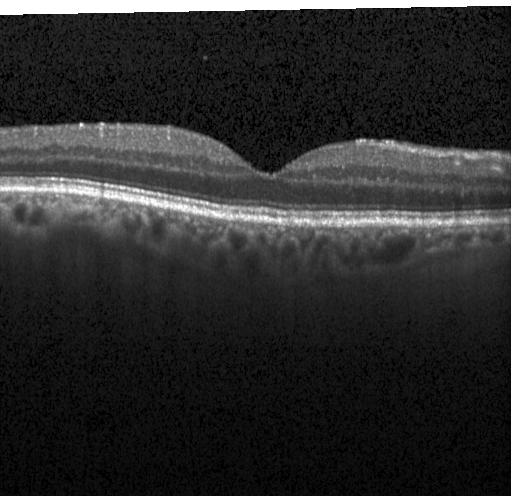 OCT B-scan showing no choroidal neovascularization, no diabetic macular edema, and no drusen.